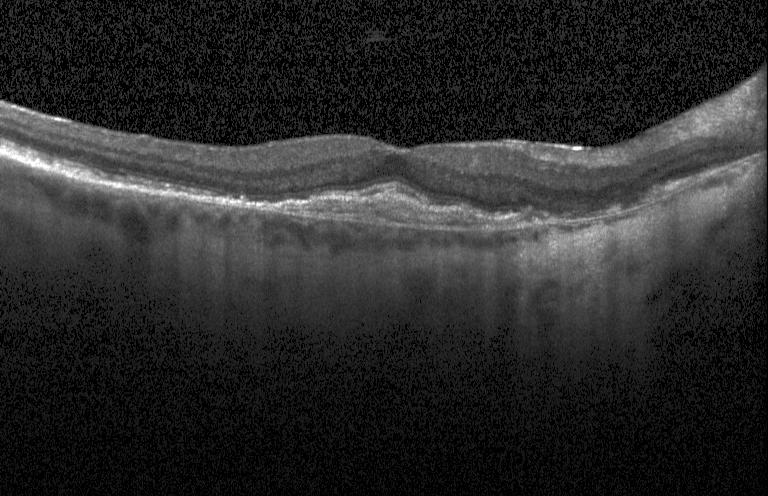
Heidelberg Spectralis, spectral-domain optical coherence tomography, retinal OCT B-scan.
Impression: a choroidal neovascular membrane.